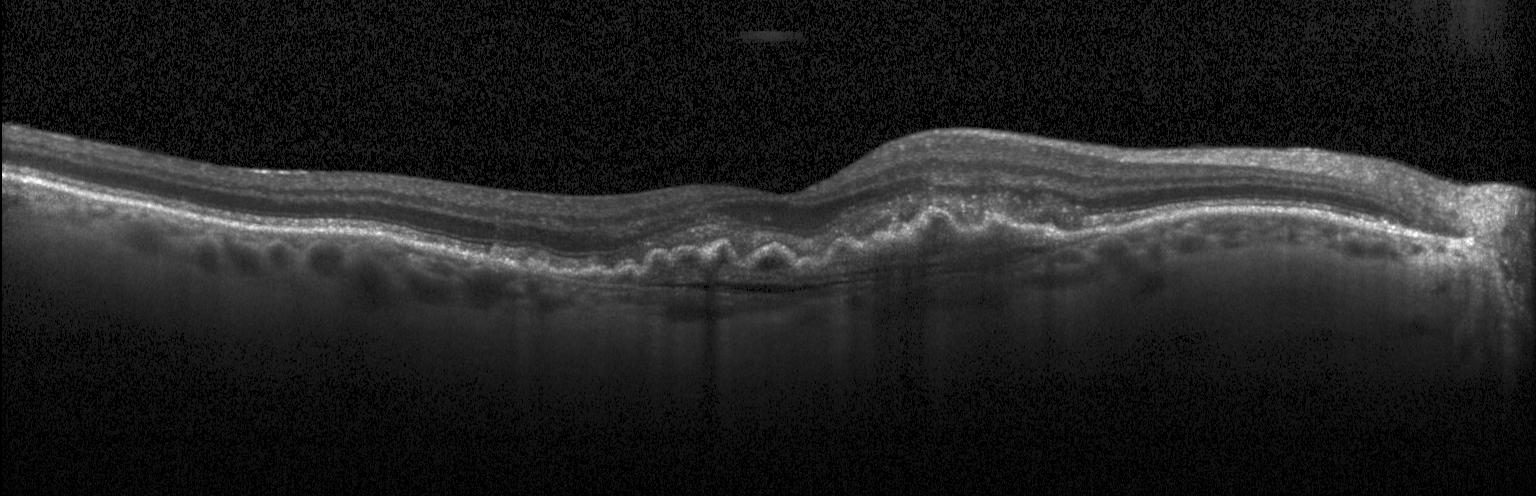
Optical coherence tomography scan. Spectral-domain optical coherence tomography. Instrument: Heidelberg Spectralis. Fovea-centered
Diagnosis: a choroidal neovascular membrane.